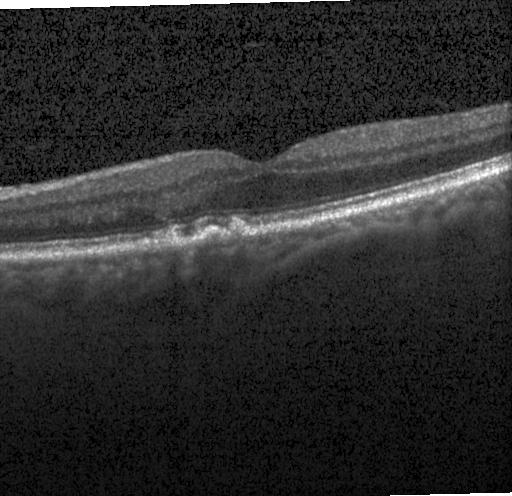
Acquired on a Heidelberg Spectralis · centered on the fovea · retinal OCT cross-section. Dx: sub-RPE drusenoid deposits.